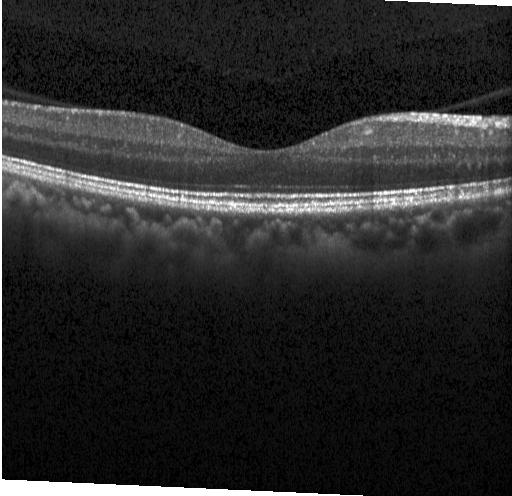
Spectral-domain OCT B-scan: no evidence of CNV, DME, or drusen.